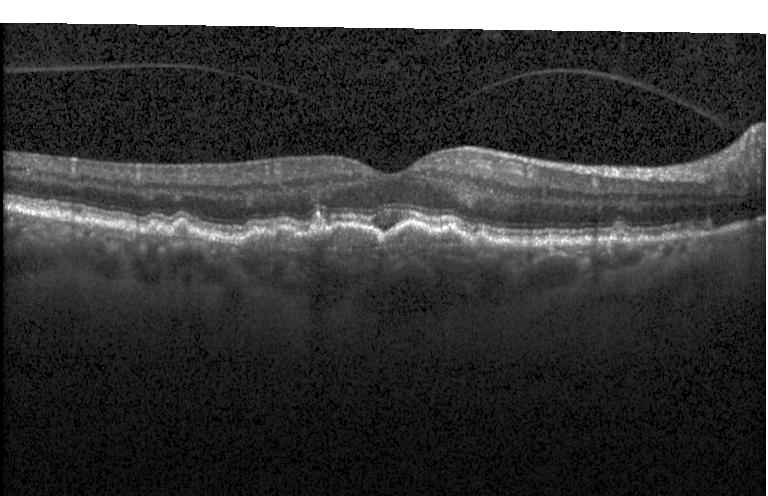
Macular OCT demonstrating a choroidal neovascular membrane.